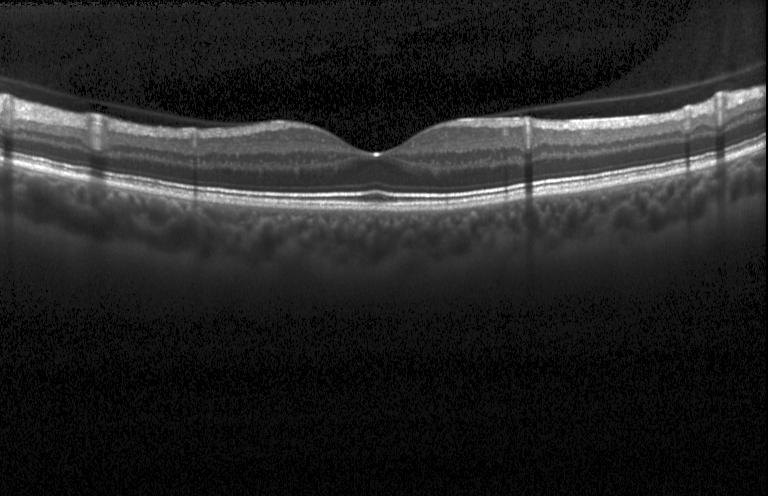

OCT line scan, instrument: Heidelberg Spectralis, horizontal scan through the fovea
Impression: no CNV, no DME, and no drusen.